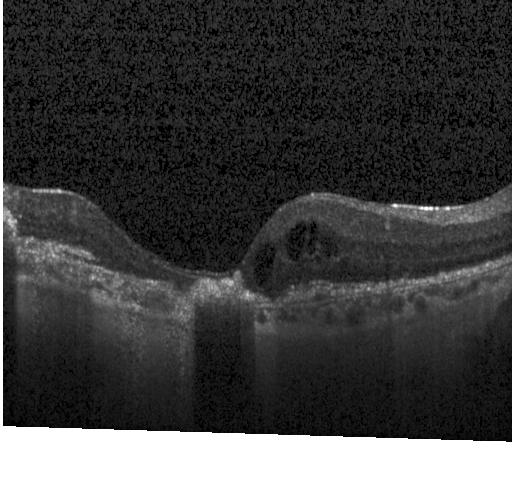

Fovea-centered, spectral-domain optical coherence tomography, retinal OCT B-scan
OCT finding: a choroidal neovascular membrane.